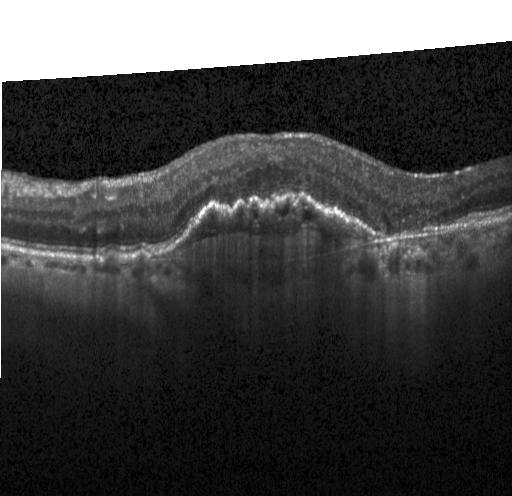
Retinal OCT cross-section. SD-OCT. Impression: choroidal neovascularization.